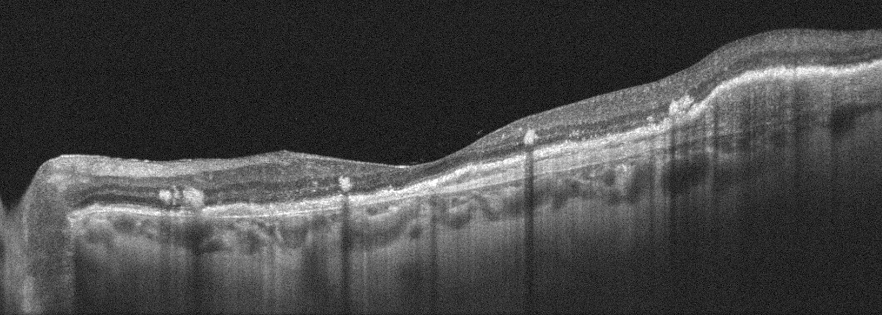
OS; retinal OCT cross-section — AMD.